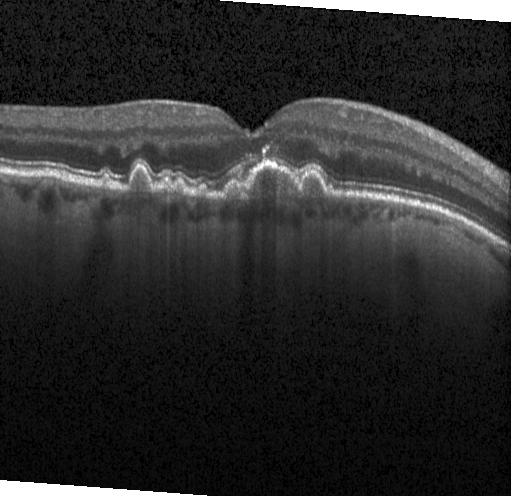 OCT B-scan showing multiple drusen.